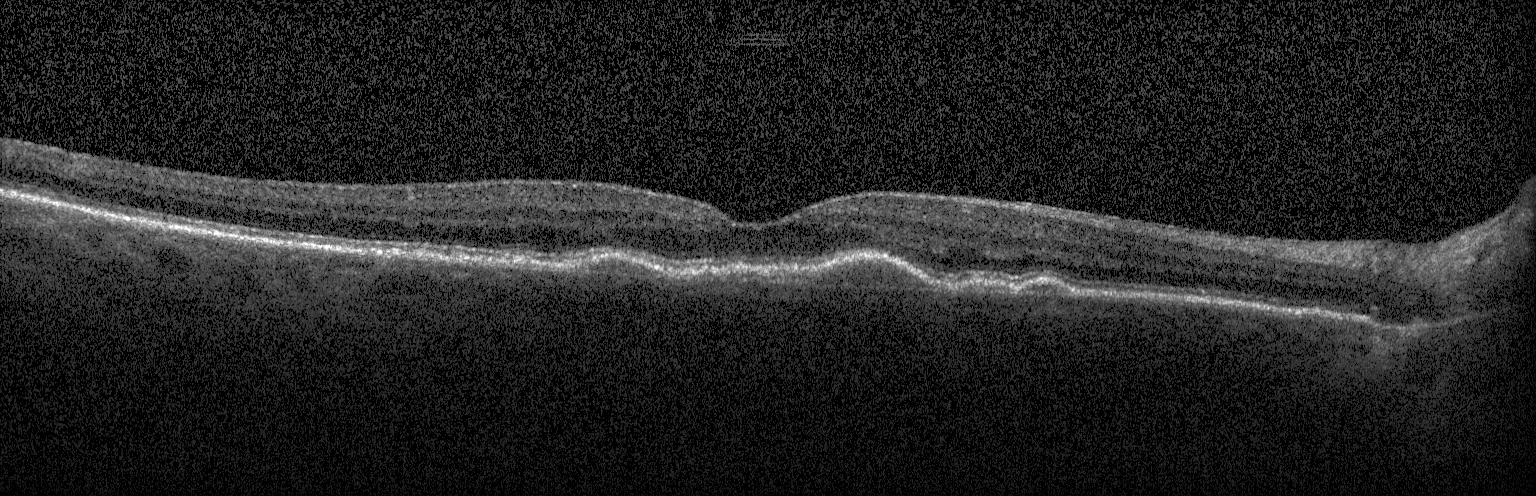
Spectral-domain optical coherence tomography. Optical coherence tomography scan — Impression: sub-RPE drusenoid deposits.